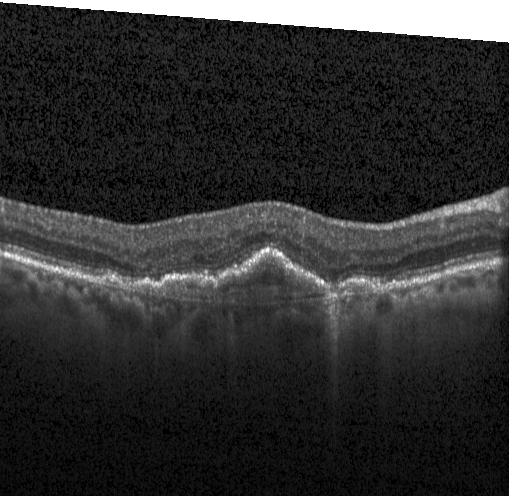 Heidelberg Spectralis OCT system; SD-OCT; centered on the fovea; retinal OCT B-scan. Impression: CNV.